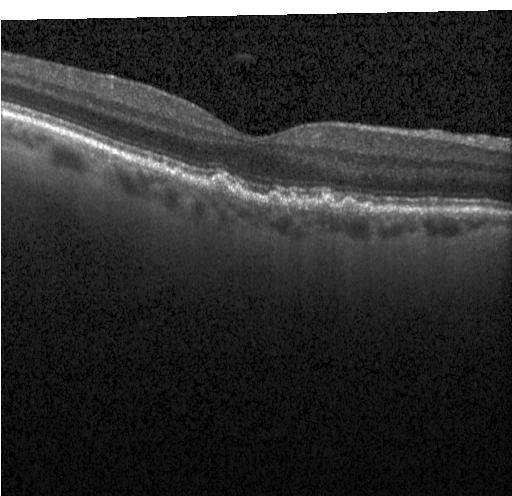
Retinal OCT B-scan · Heidelberg Spectralis · spectral-domain OCT · macular scan
Impression: multiple drusen.